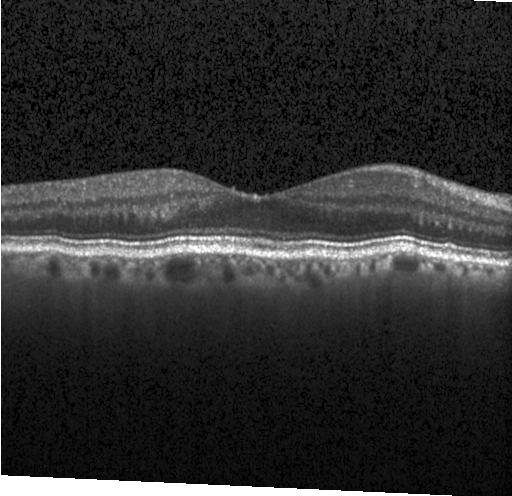 Optical coherence tomography B-scan
Impression: no choroidal neovascularization, diabetic macular edema, or drusen.